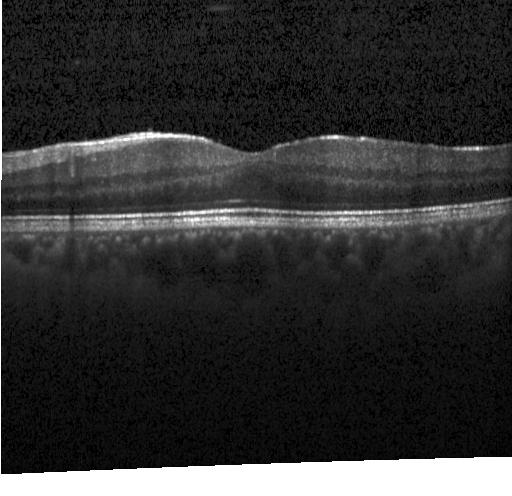

Optical coherence tomography B-scan. Spectral-domain optical coherence tomography. Through the macula — Neither choroidal neovascularization, diabetic macular edema, nor drusen.